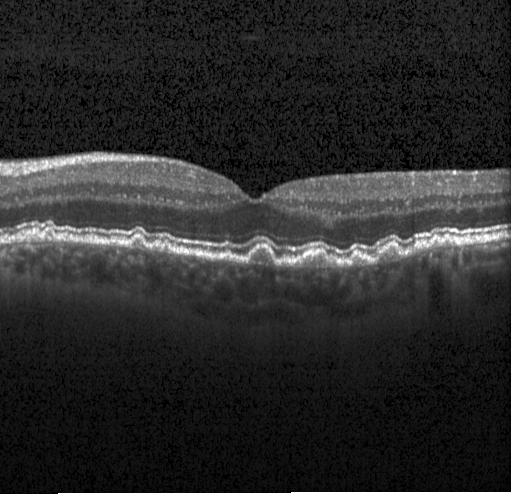 Horizontal scan through the fovea. Retinal OCT B-scan. Heidelberg Spectralis
Diagnosis: multiple drusen.